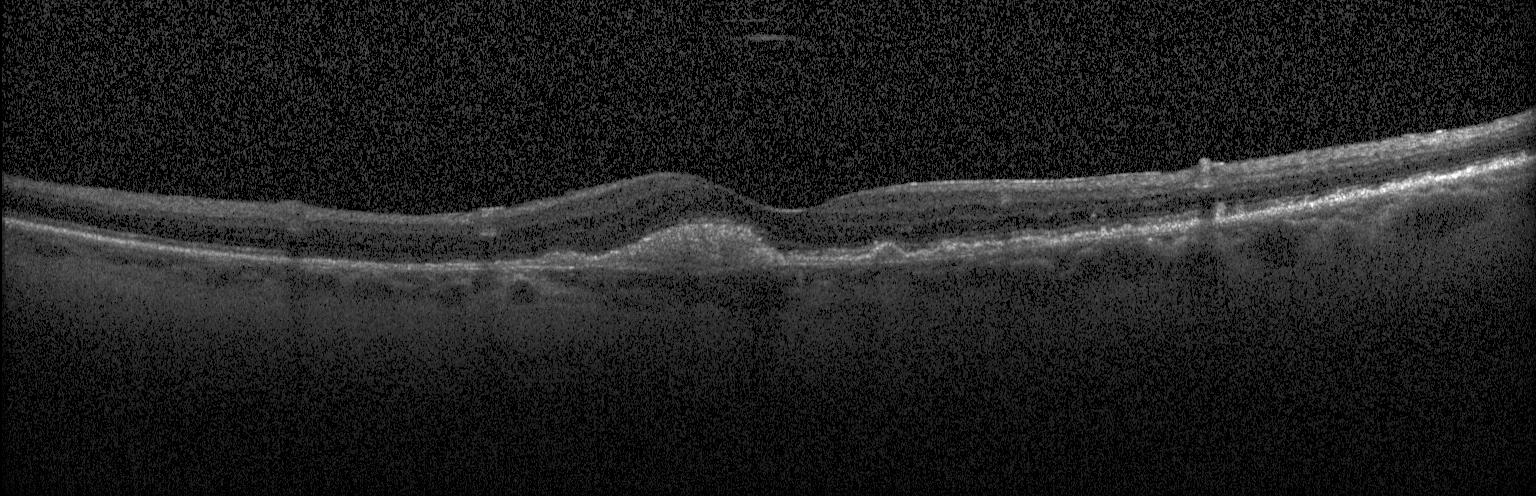

Optical coherence tomography scan — A choroidal neovascular membrane.